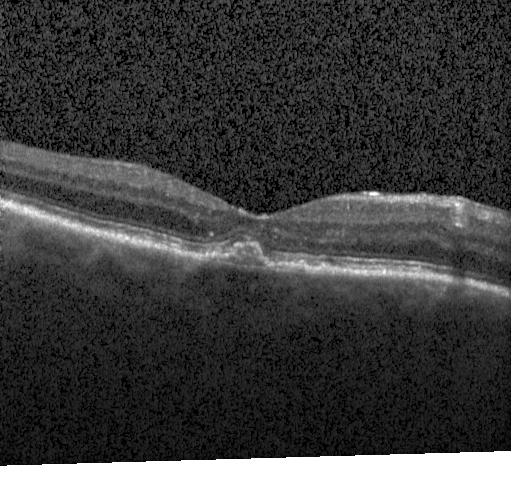
SD-OCT. Retinal OCT B-scan. Fovea-centered
This B-scan demonstrates a choroidal neovascular membrane.